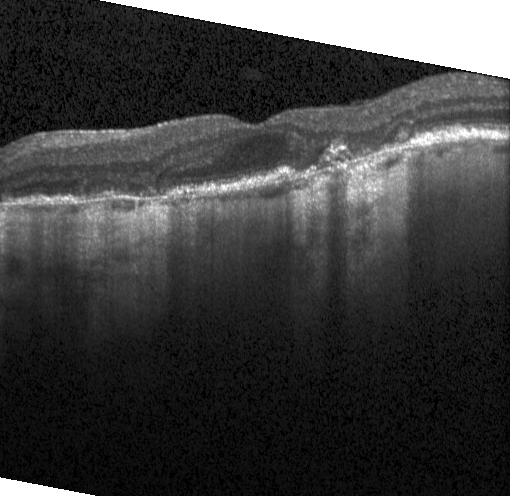

Centered on the fovea, optical coherence tomography scan, SD-OCT
Assessment: CNV.